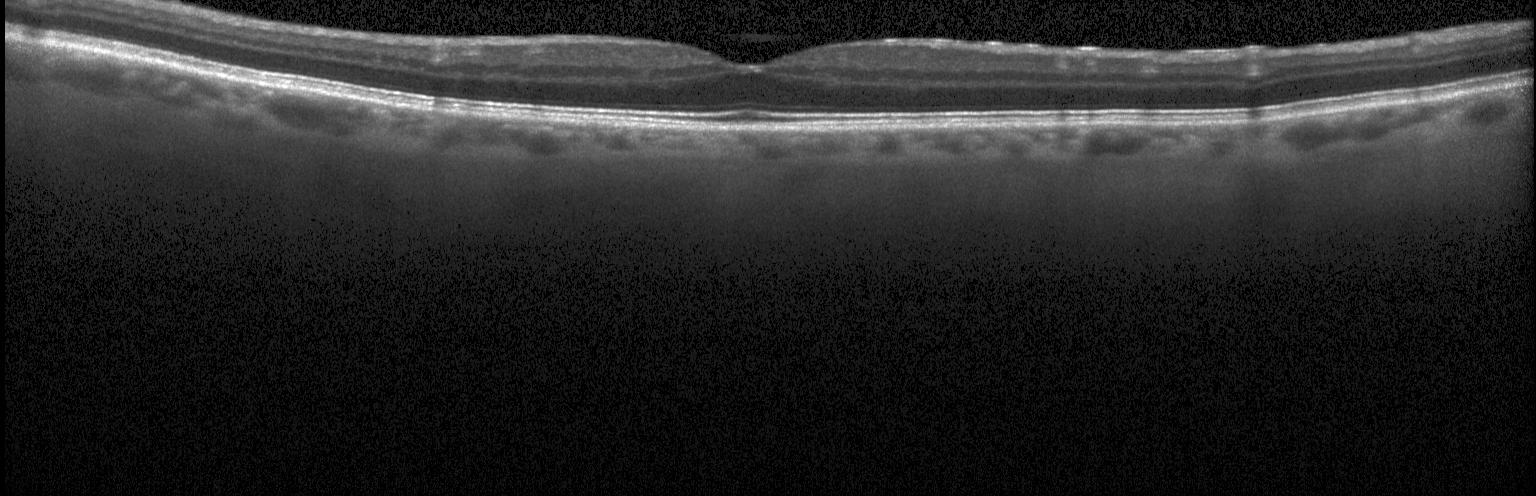

This B-scan demonstrates no evidence of choroidal neovascularization, diabetic macular edema, or drusen.